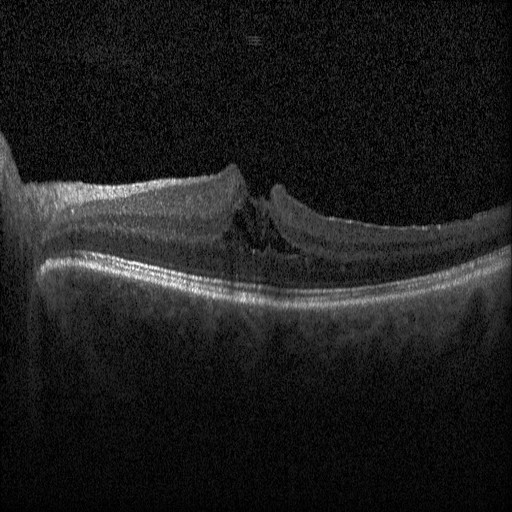
Diagnosis: diabetic macular edema.